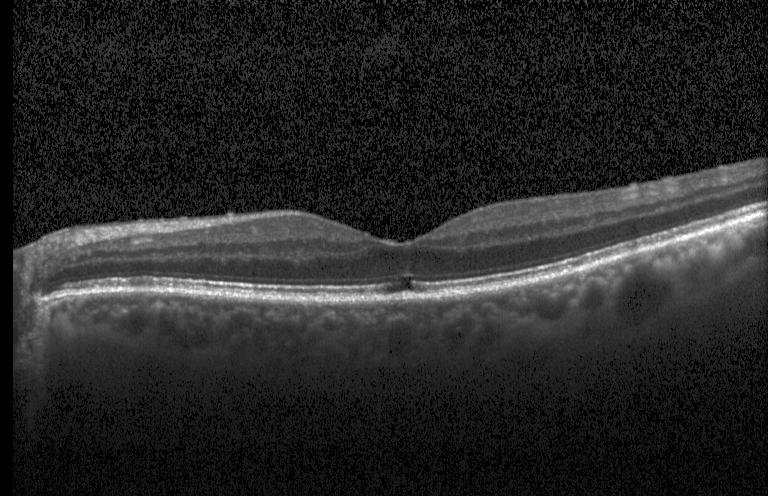
Retinal OCT B-scan — Dx: no CNV, DME, or drusen.